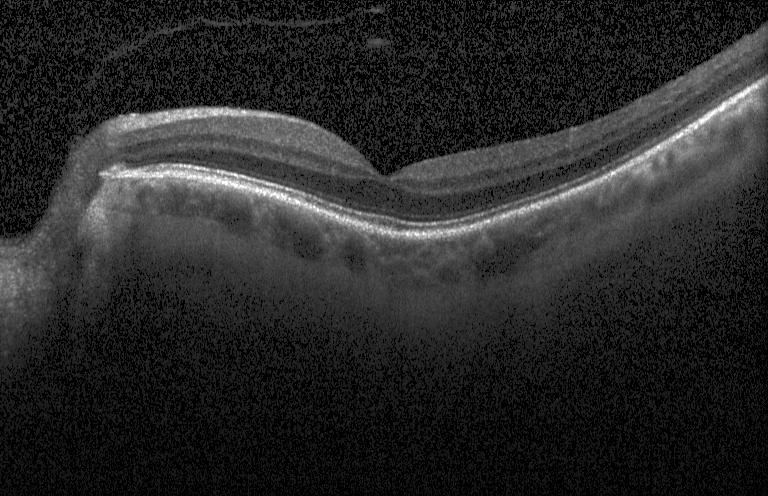
Fovea-centered. Optical coherence tomography B-scan.
Finding: no CNV, DME, or drusen.